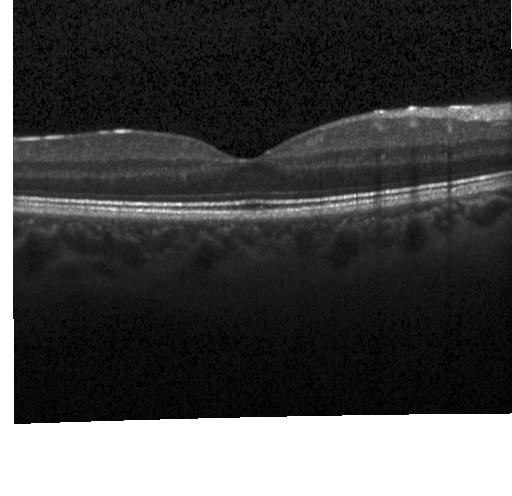 Macular OCT: no CNV, no DME, and no drusen.